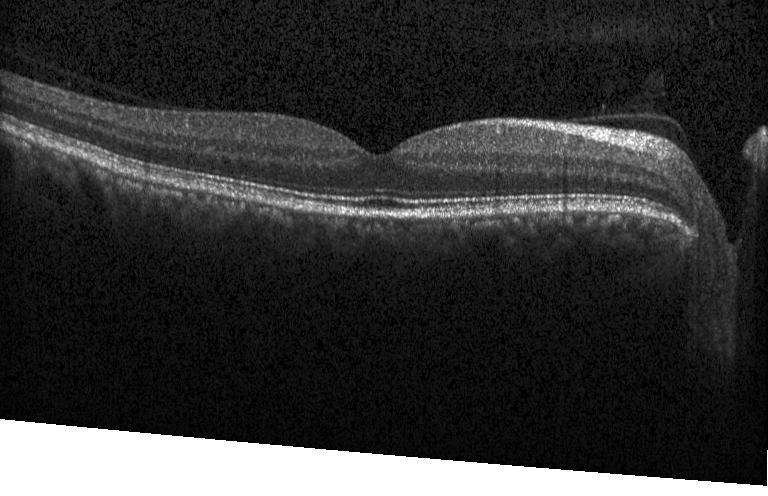
Through the macula, retinal OCT B-scan
Impression: no evidence of choroidal neovascularization, diabetic macular edema, or drusen.